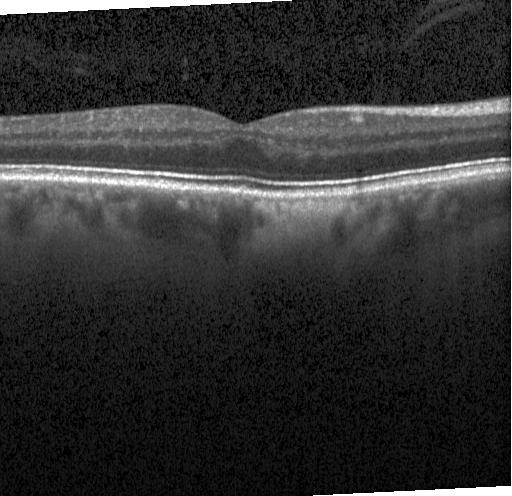

Heidelberg Spectralis OCT system. Horizontal scan through the fovea. SD-OCT. OCT B-scan — The scan shows no evidence of choroidal neovascularization, diabetic macular edema, or drusen.